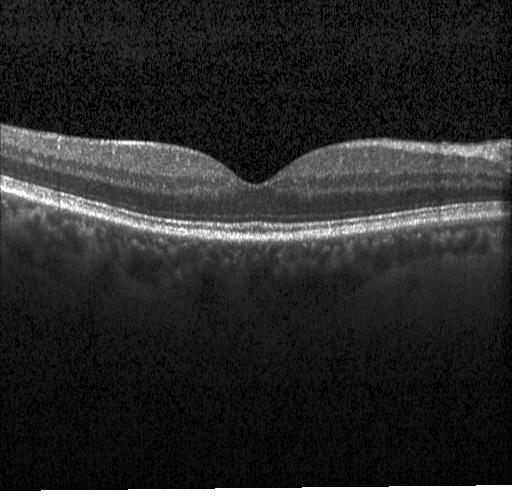
Spectral-domain OCT. Horizontal scan through the fovea. Heidelberg Spectralis OCT system. Optical coherence tomography scan. Assessment: no choroidal neovascularization, diabetic macular edema, or drusen.